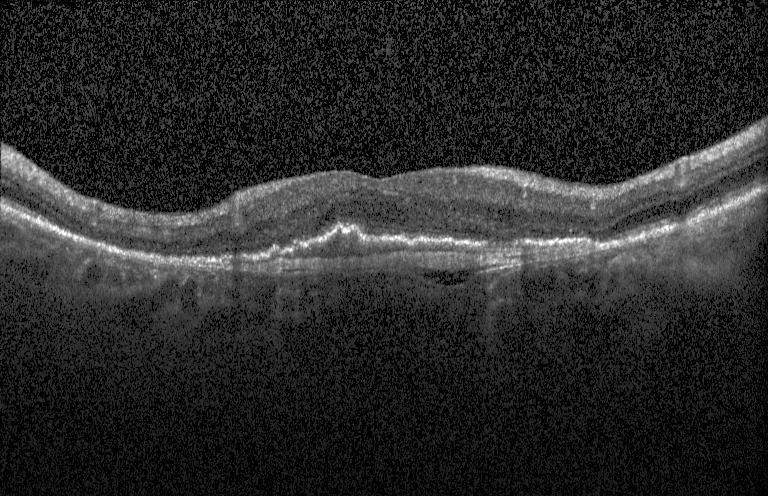 Through the macula. Spectral-domain OCT. OCT line scan. The scan shows CNV.